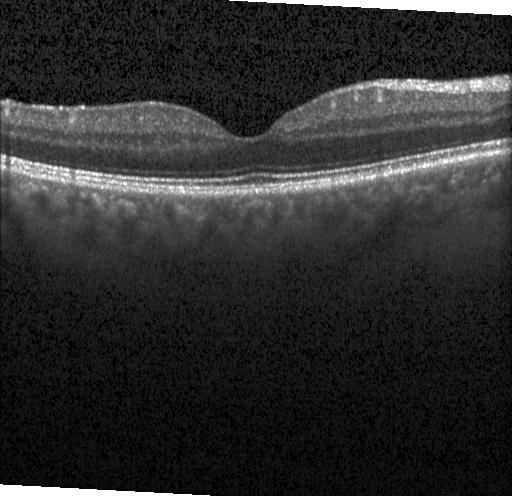
Instrument: Heidelberg Spectralis, optical coherence tomography scan, through the macula, spectral-domain optical coherence tomography — Impression: no choroidal neovascularization, no diabetic macular edema, and no drusen.